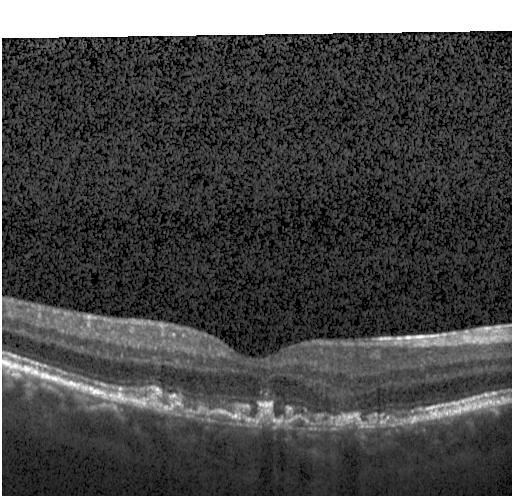

Optical coherence tomography scan. The scan shows CNV.